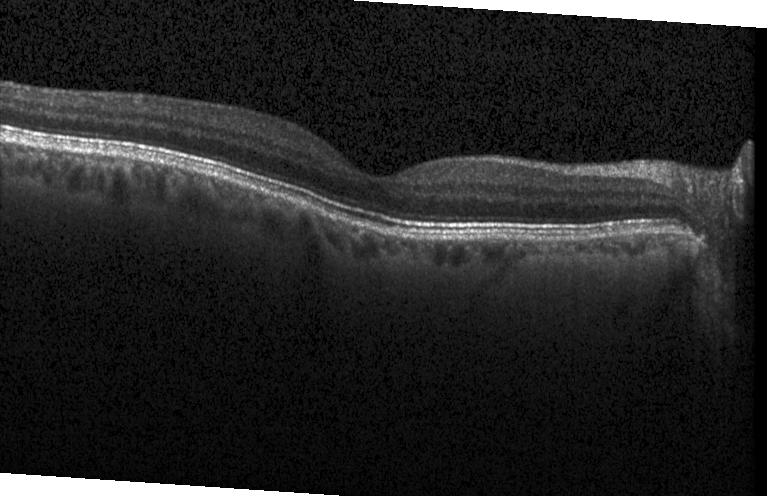
Retinal OCT cross-section showing no evidence of choroidal neovascularization, diabetic macular edema, or drusen.